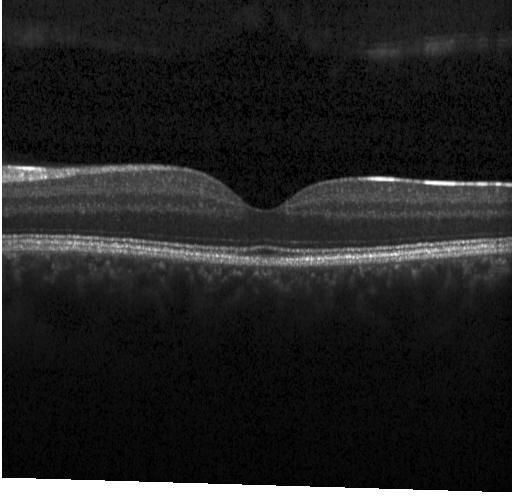 OCT B-scan · Heidelberg Spectralis OCT system — Finding: no evidence of choroidal neovascularization, diabetic macular edema, or drusen.